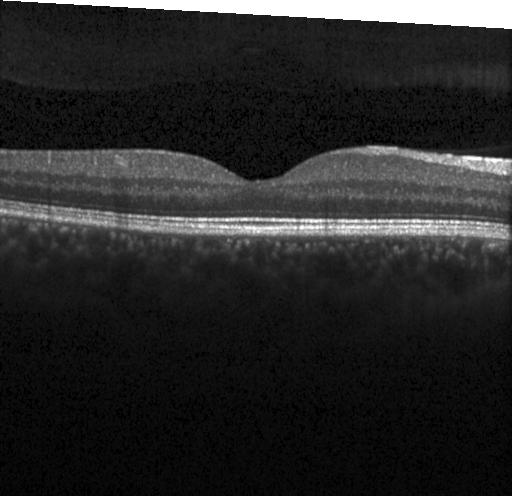
OCT scan showing no choroidal neovascularization, diabetic macular edema, or drusen.